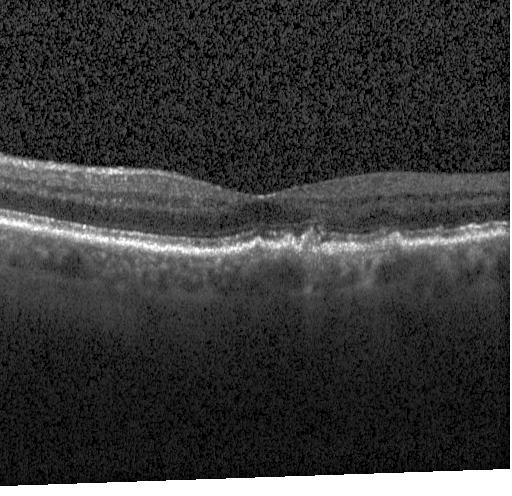
Fovea-centered · retinal OCT B-scan · spectral-domain OCT — Diagnosis: multiple drusen.